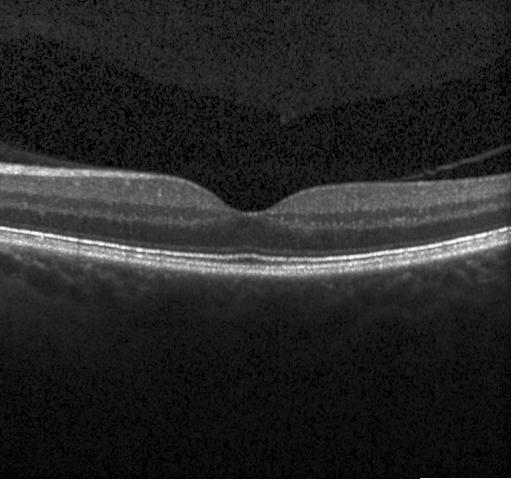
Finding: neither choroidal neovascularization, diabetic macular edema, nor drusen.